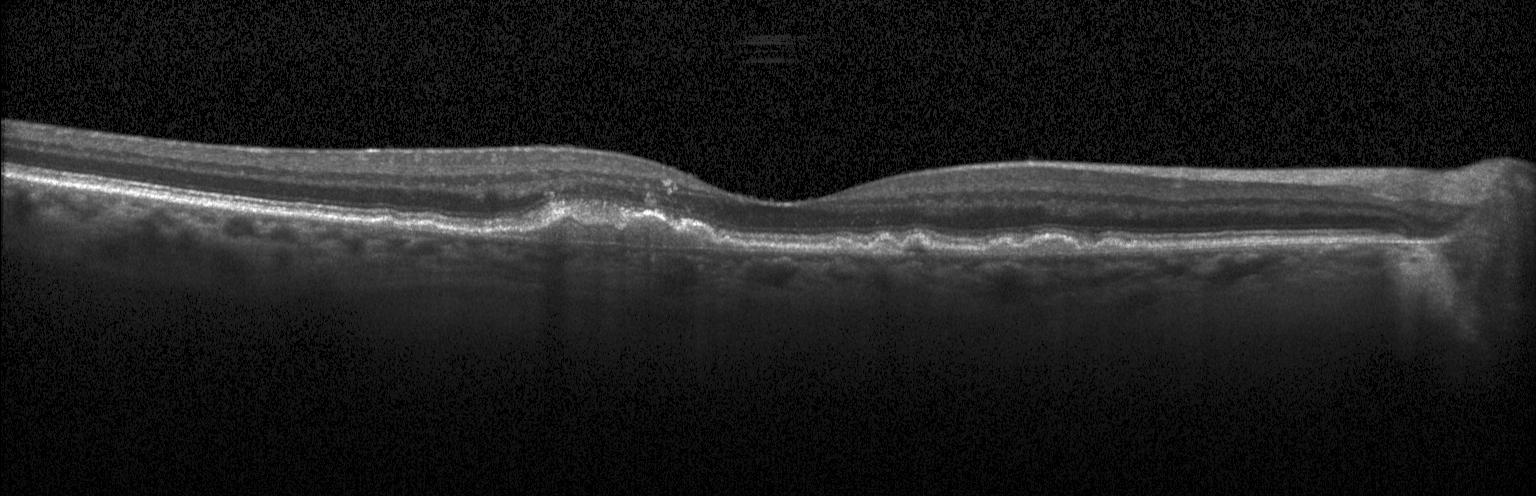

Finding: a choroidal neovascular membrane.